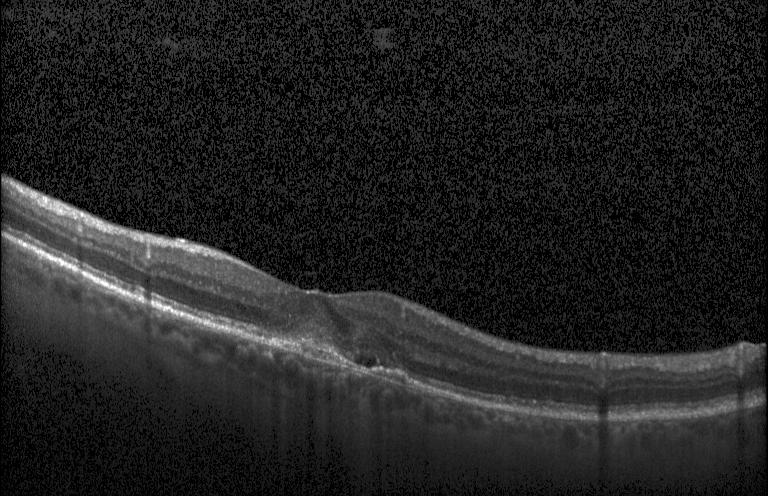
Centered on the fovea. SD-OCT. OCT B-scan. Instrument: Heidelberg Spectralis. The scan shows choroidal neovascularization.